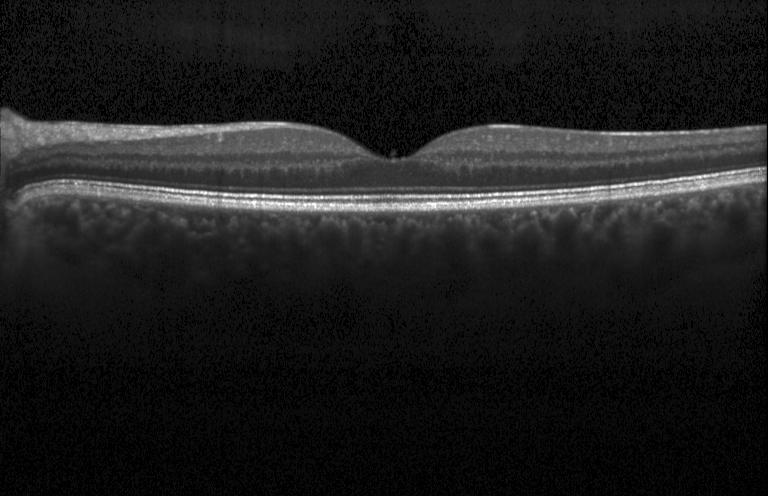 OCT line scan. Centered on the fovea. Instrument: Heidelberg Spectralis — No choroidal neovascularization, no diabetic macular edema, and no drusen.